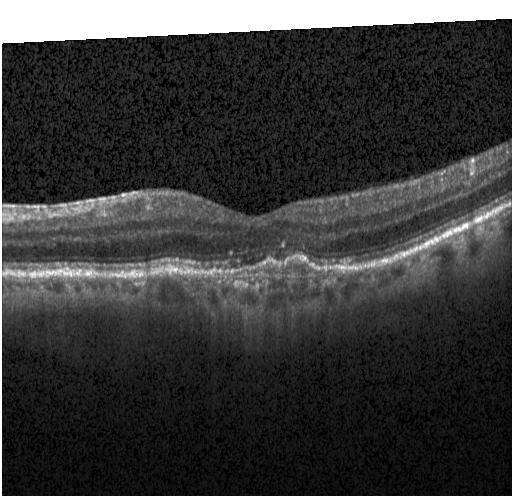

Retinal OCT cross-section, spectral-domain optical coherence tomography — Impression: a choroidal neovascular membrane.